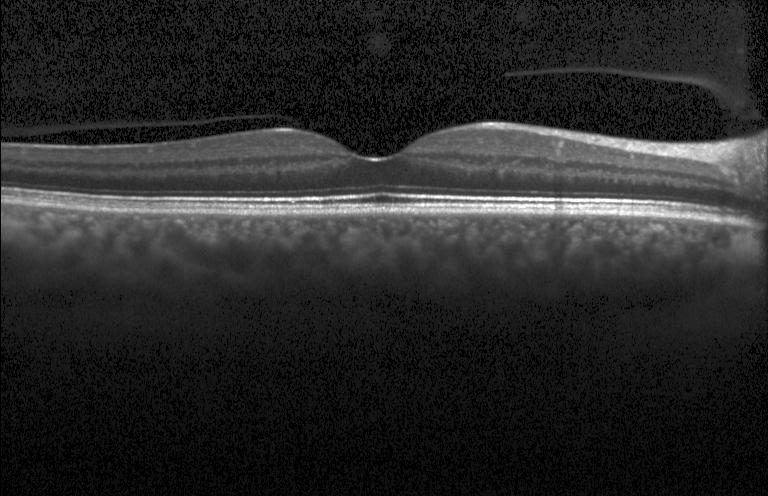
Finding: neither choroidal neovascularization, diabetic macular edema, nor drusen.